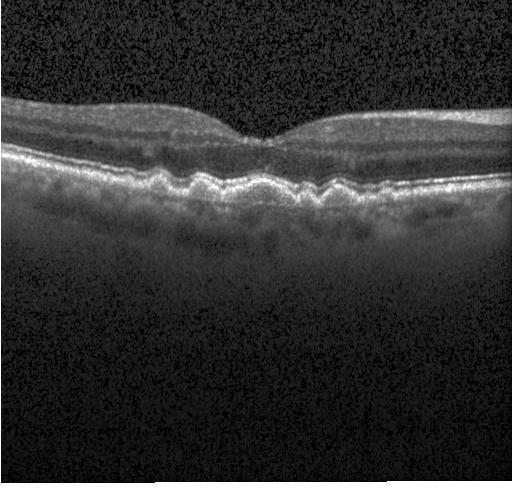

OCT B-scan showing sub-RPE drusenoid deposits.